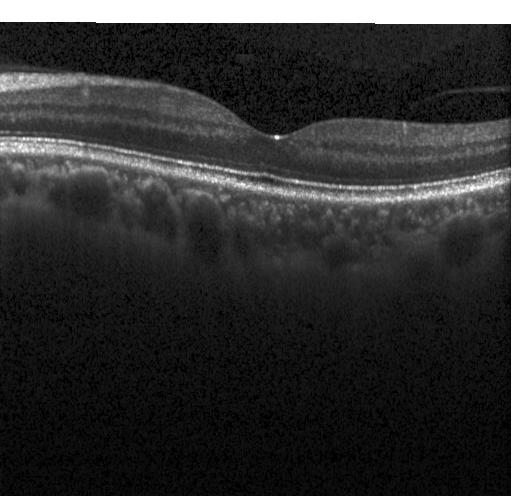

Heidelberg Spectralis OCT system. Optical coherence tomography B-scan. Fovea-centered.
OCT finding: no CNV, DME, or drusen.